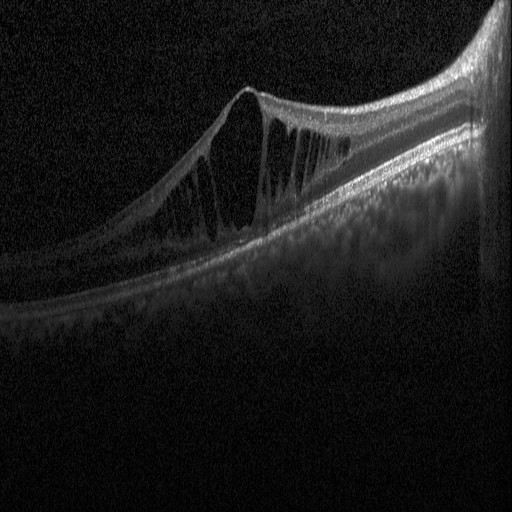 OCT B-scan, macular scan
Diagnosis: diabetic macular edema (DME).